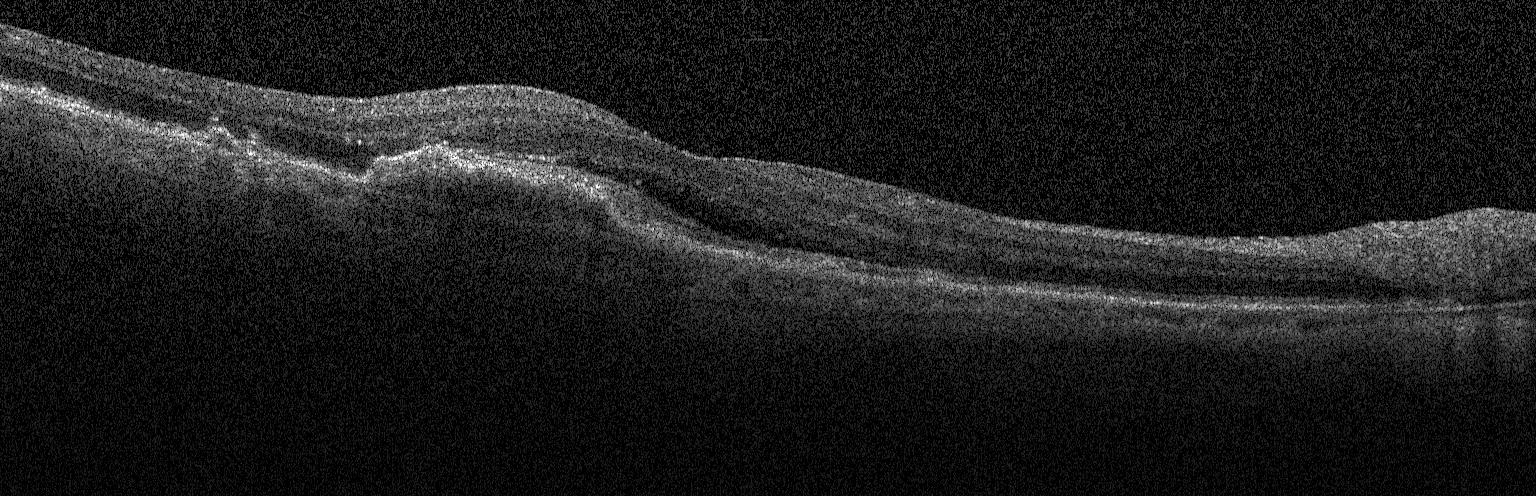 OCT line scan — Finding: choroidal neovascularization.